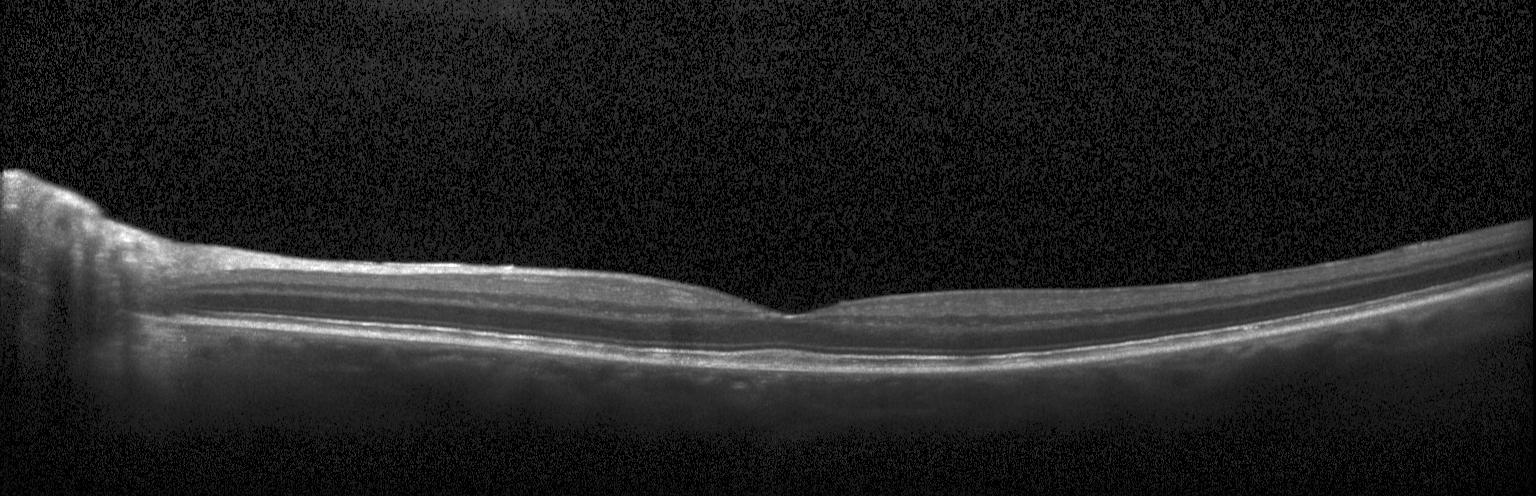 Impression: no choroidal neovascularization, diabetic macular edema, or drusen.